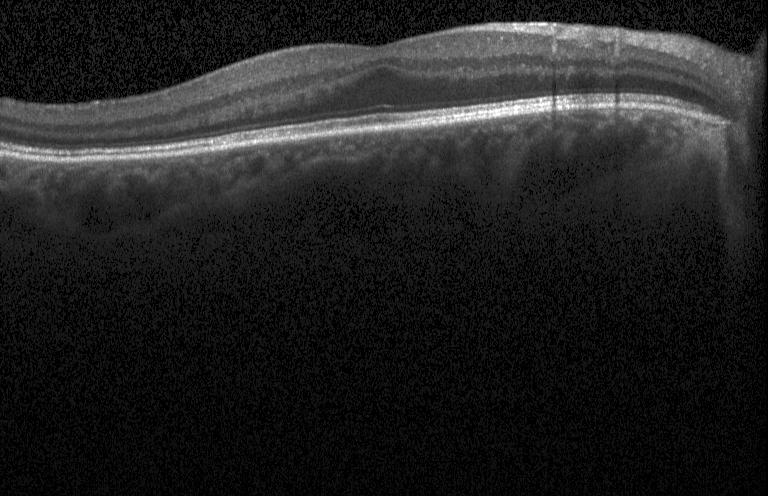
Spectral-domain OCT; retinal OCT B-scan; macular scan — This B-scan demonstrates neither choroidal neovascularization, diabetic macular edema, nor drusen.